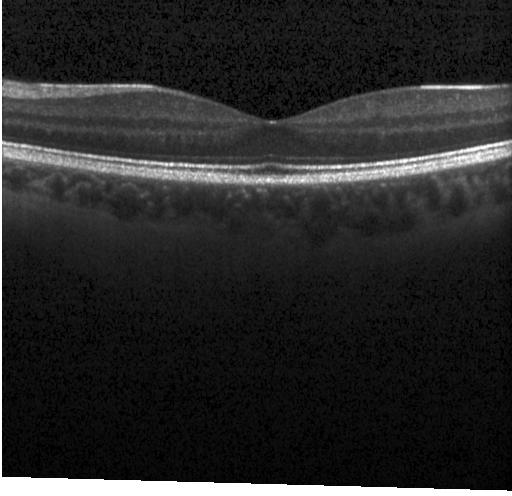

Dx: neither choroidal neovascularization, diabetic macular edema, nor drusen.